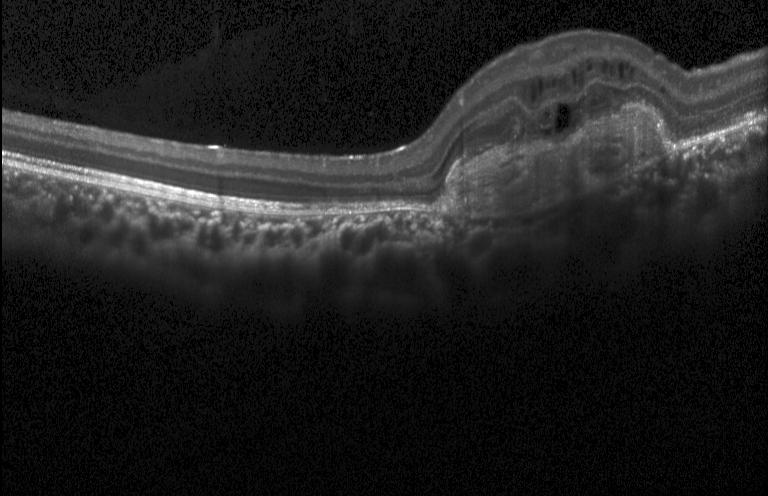

Retinal OCT cross-section, through the macula
Diagnosis: a choroidal neovascular membrane.